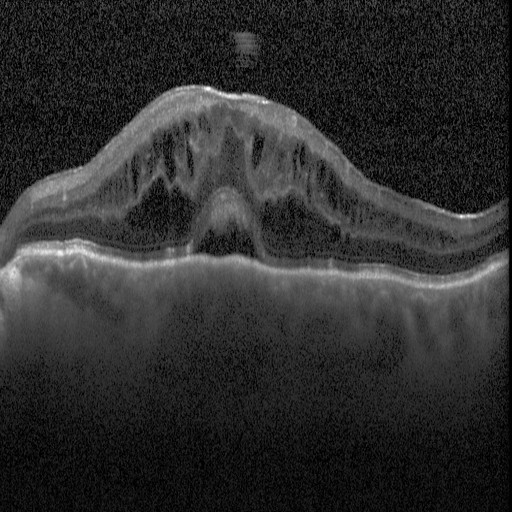
Horizontal scan through the fovea · acquired on a Heidelberg Spectralis · SD-OCT · retinal OCT B-scan
Diagnosis: DME.